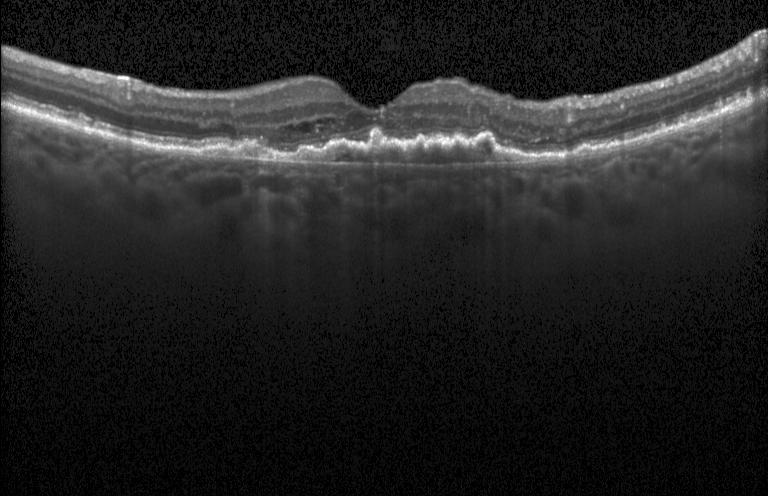 Horizontal scan through the fovea, retinal OCT cross-section, acquired on a Heidelberg Spectralis
This B-scan demonstrates choroidal neovascularization.